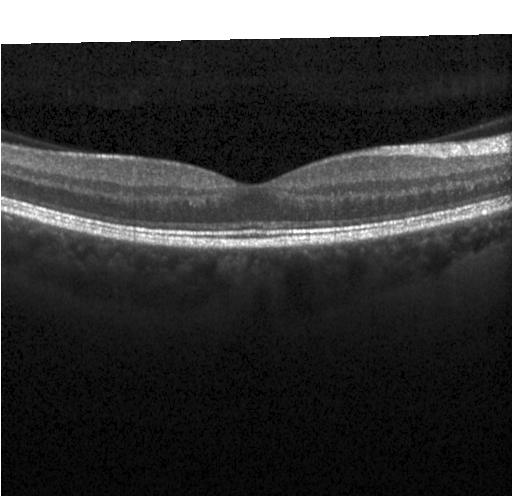 Finding: no CNV, DME, or drusen.